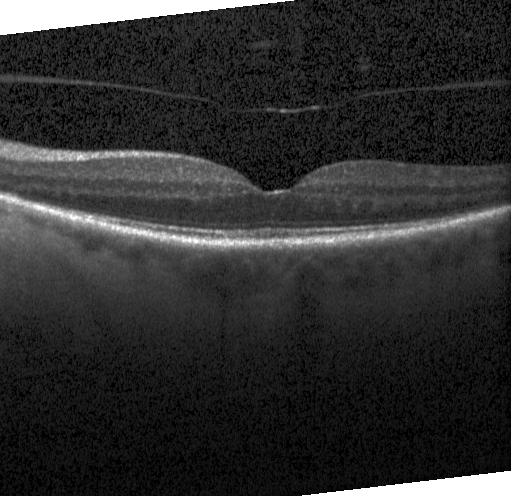

OCT finding: no evidence of CNV, DME, or drusen.